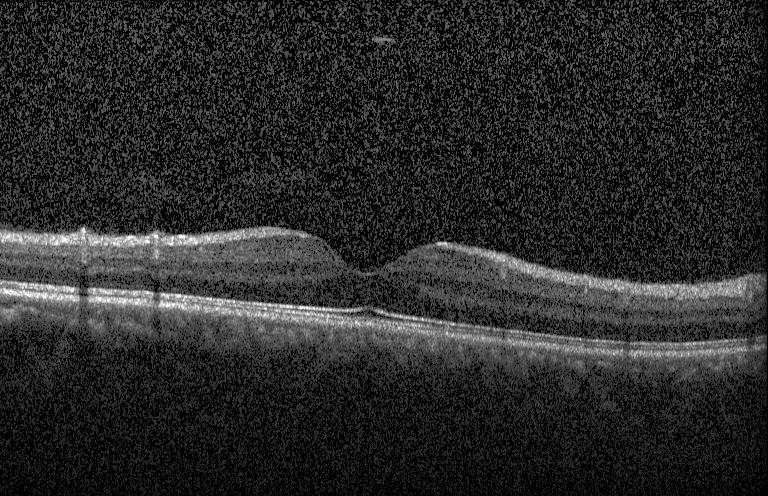 No evidence of choroidal neovascularization, diabetic macular edema, or drusen.